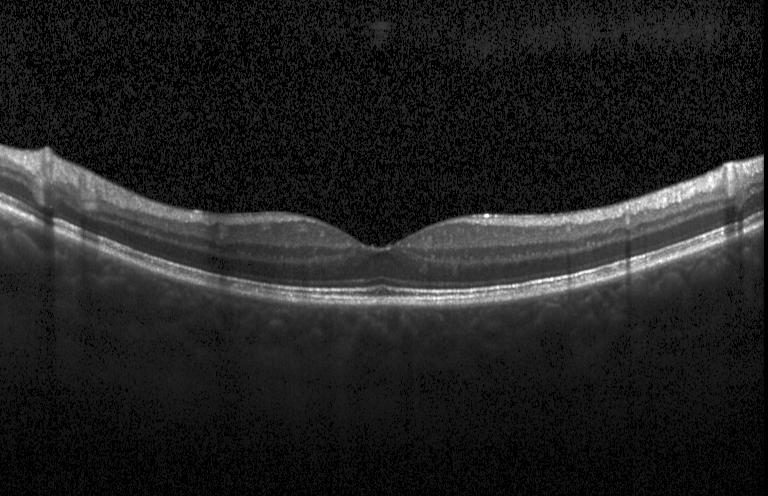 Retinal OCT B-scan — Macular OCT: neither choroidal neovascularization, diabetic macular edema, nor drusen.